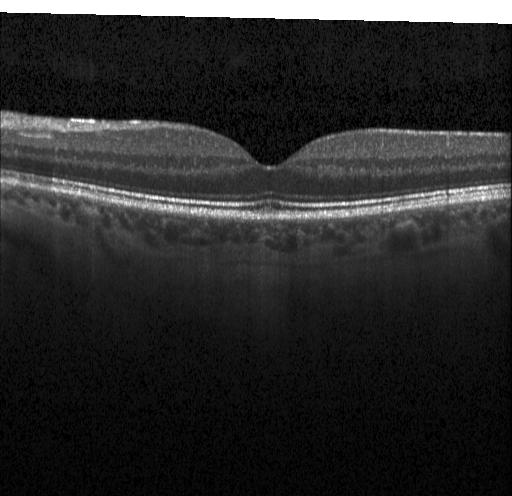
Spectral-domain OCT B-scan: no choroidal neovascularization, no diabetic macular edema, and no drusen.